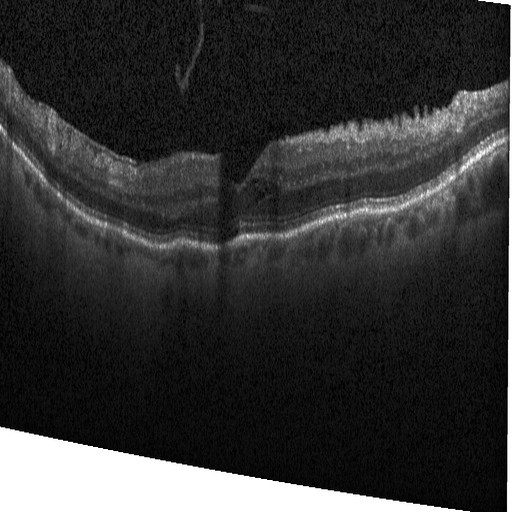

Finding: DME.